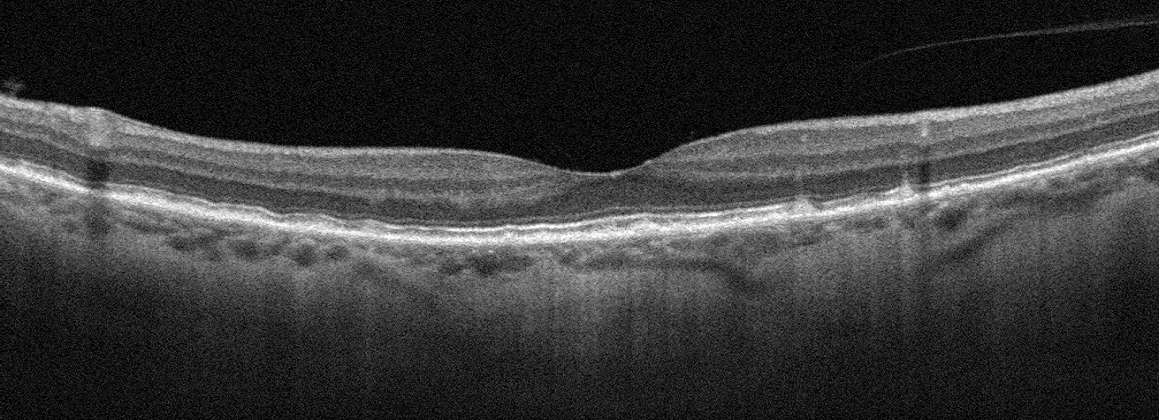

OS · macular scan · Optovue Avanti RTVue XR · retinal OCT B-scan. The scan shows AMD.